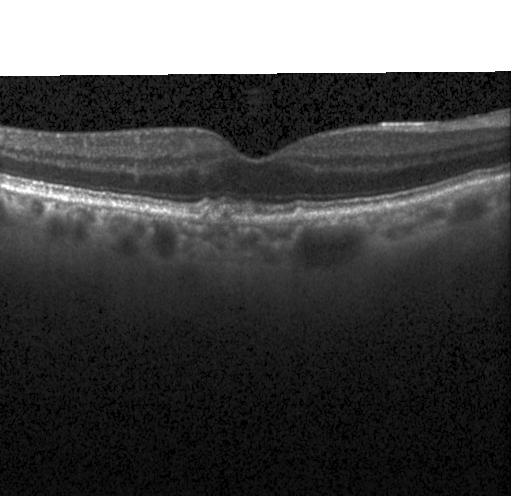

OCT scan showing sub-RPE drusenoid deposits.